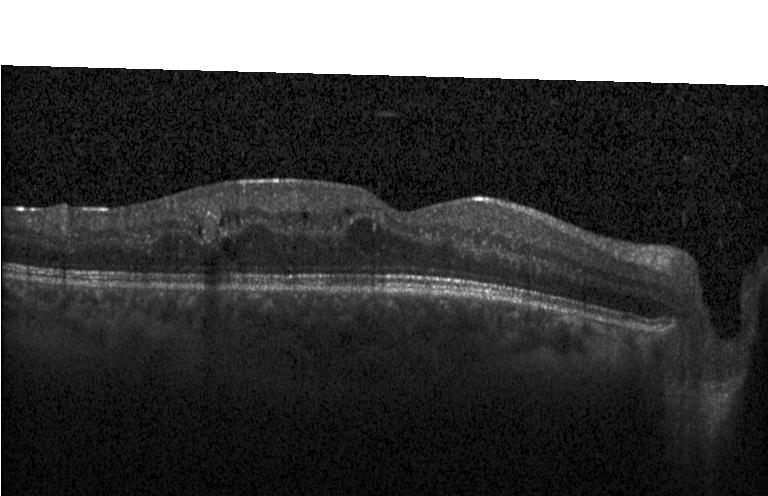

Finding: DME.